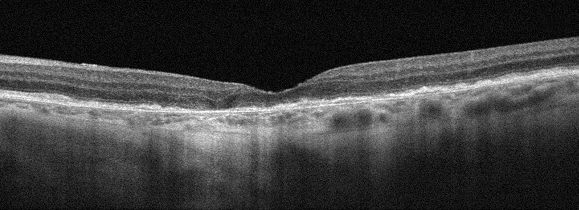

OS. Optovue Avanti RTVue XR. Optical coherence tomography scan.
Impression: AMD.